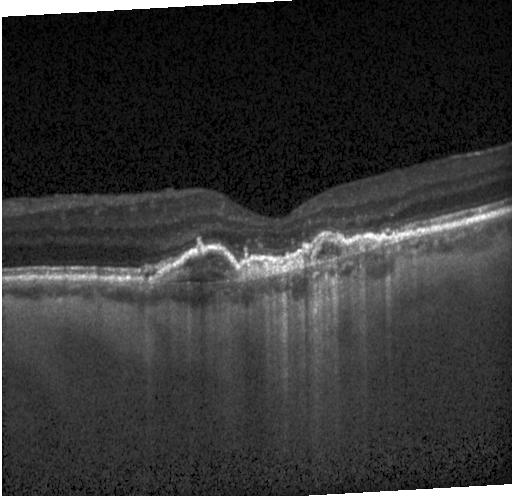
Diagnosis: choroidal neovascularization.